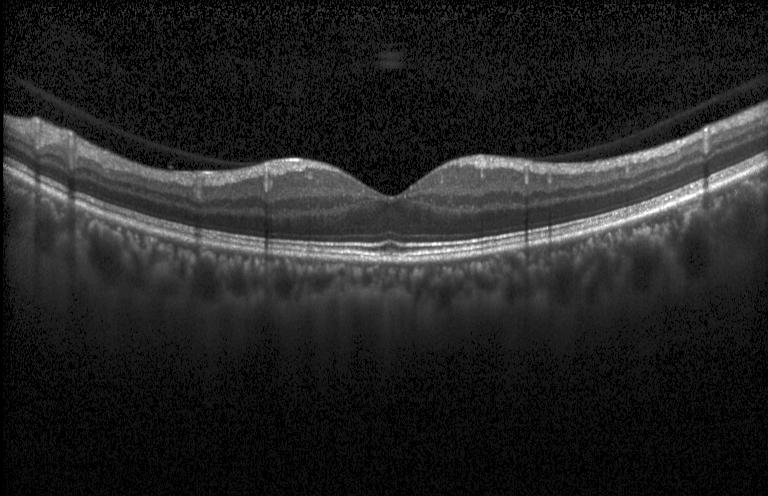

Horizontal scan through the fovea · optical coherence tomography scan.
Impression: neither choroidal neovascularization, diabetic macular edema, nor drusen.